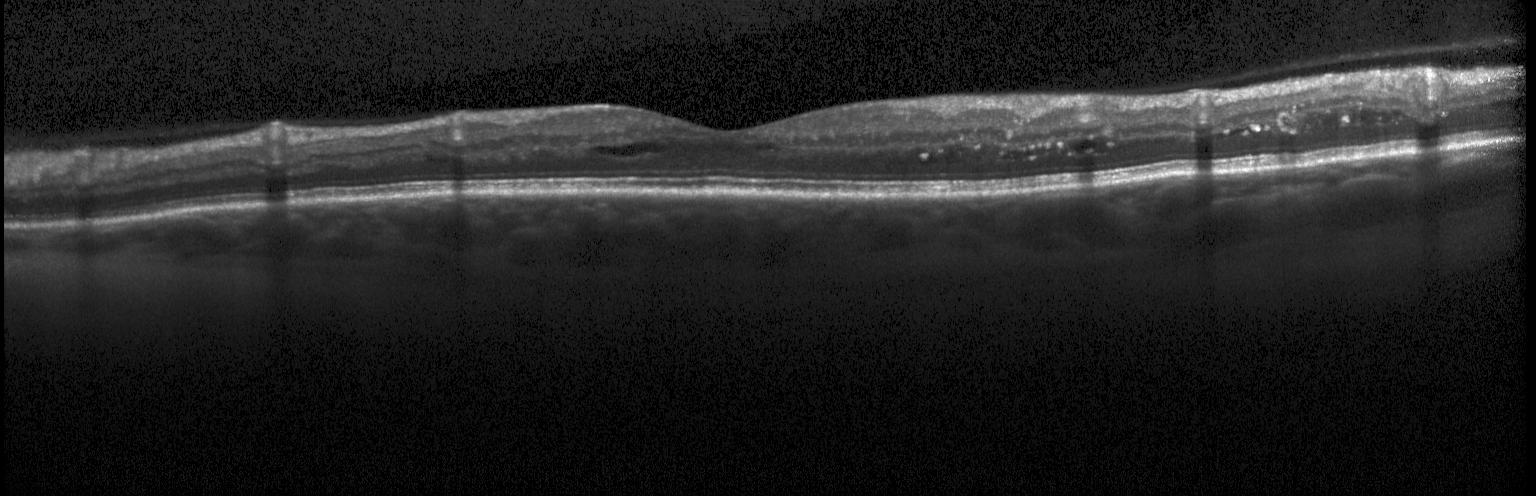 Retinal OCT cross-section, spectral-domain OCT
OCT finding: diabetic macular edema (DME).